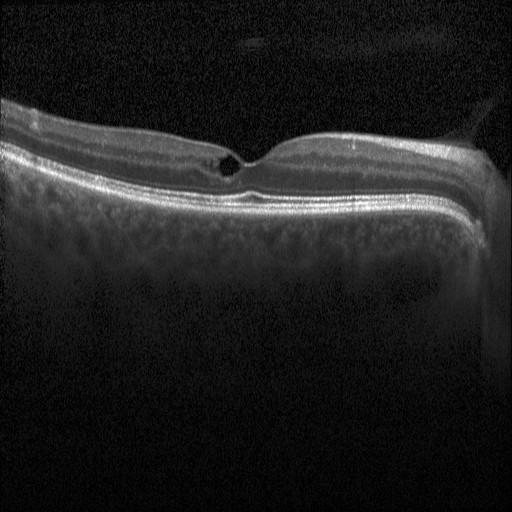
Centered on the fovea · OCT B-scan · acquired on a Heidelberg Spectralis · SD-OCT.
Assessment: DME.